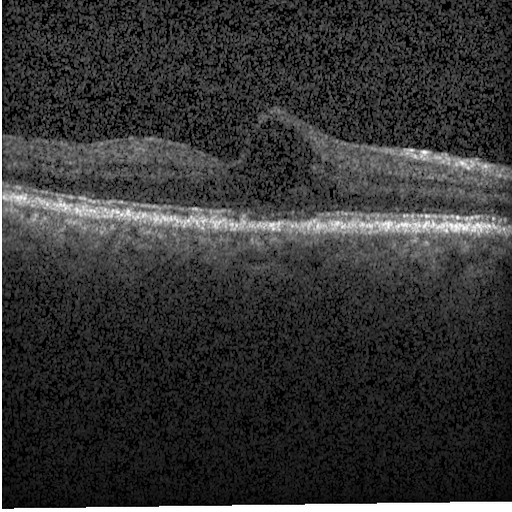 OCT line scan
Dx: diabetic macular edema.